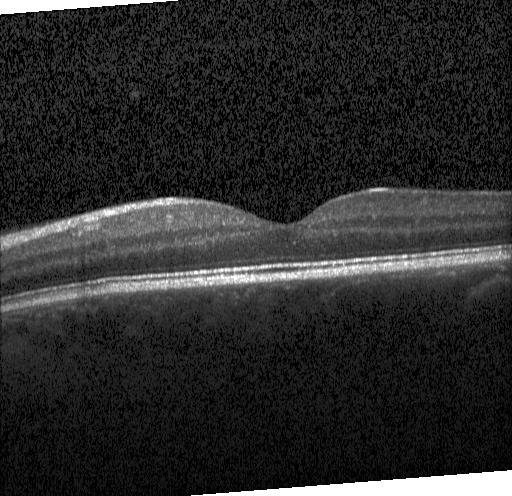 Diagnosis: no CNV, no DME, and no drusen.